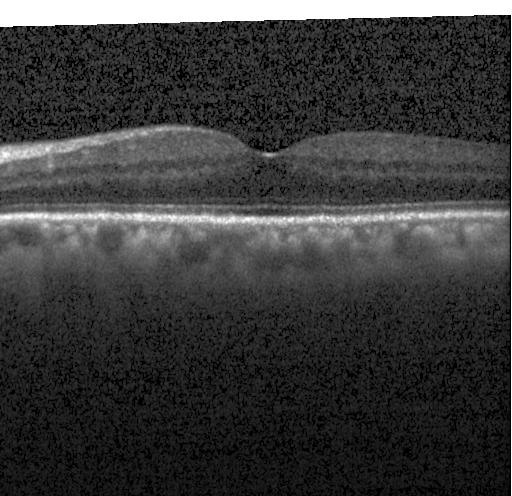

Heidelberg Spectralis OCT system. Retinal OCT B-scan.
Finding: neither choroidal neovascularization, diabetic macular edema, nor drusen.